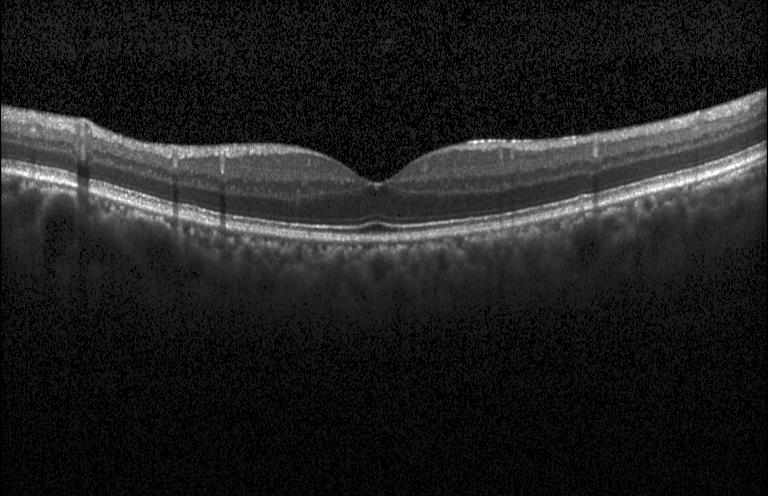

Macular OCT demonstrating no choroidal neovascularization, no diabetic macular edema, and no drusen.